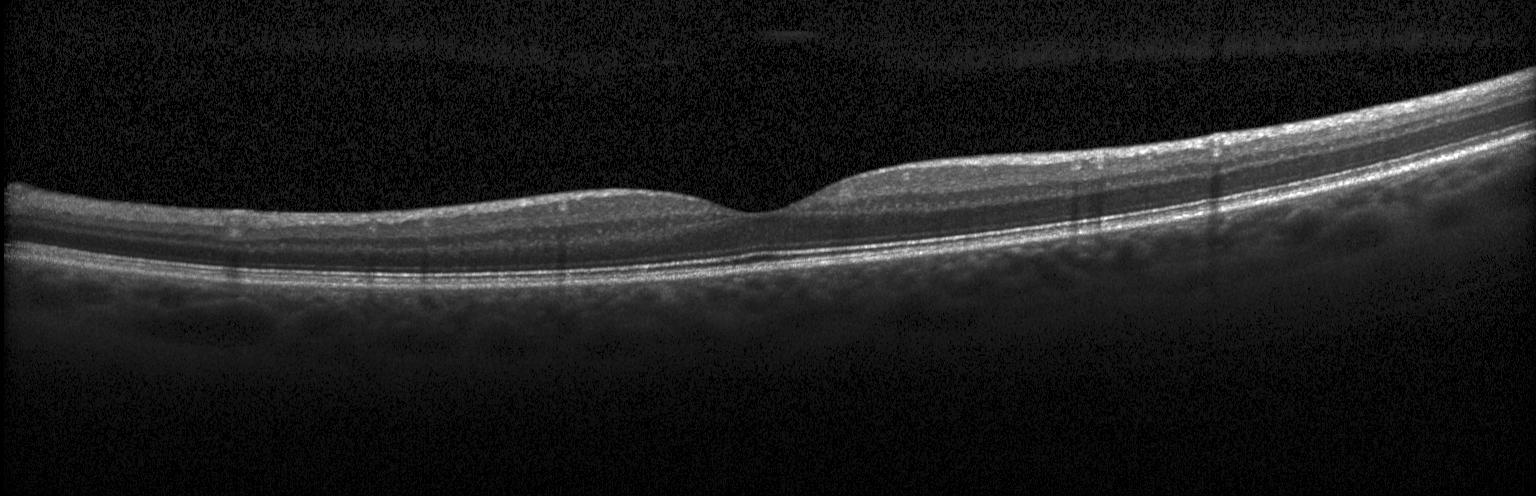
Diagnosis: no evidence of choroidal neovascularization, diabetic macular edema, or drusen.